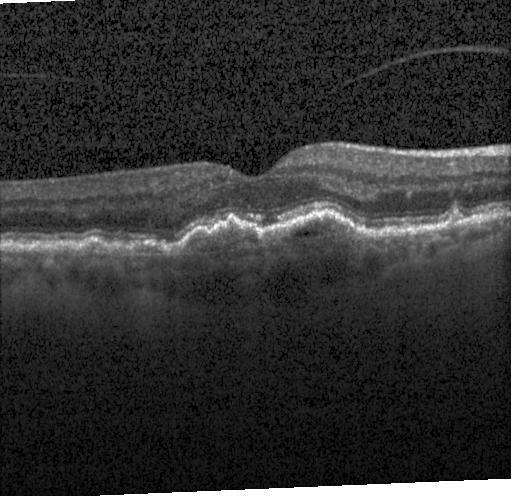 Retinal OCT B-scan. Macular scan
The scan shows CNV.